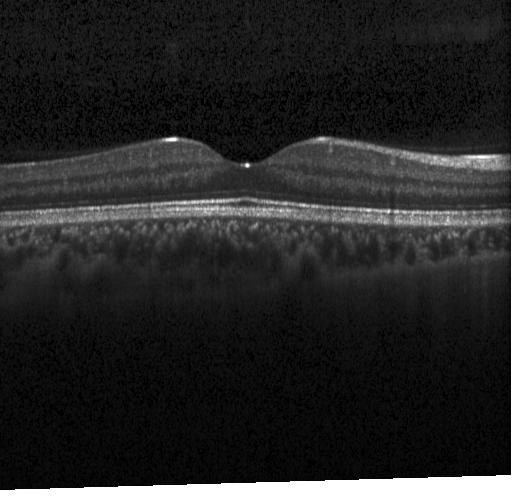 OCT line scan — Finding: no CNV, DME, or drusen.